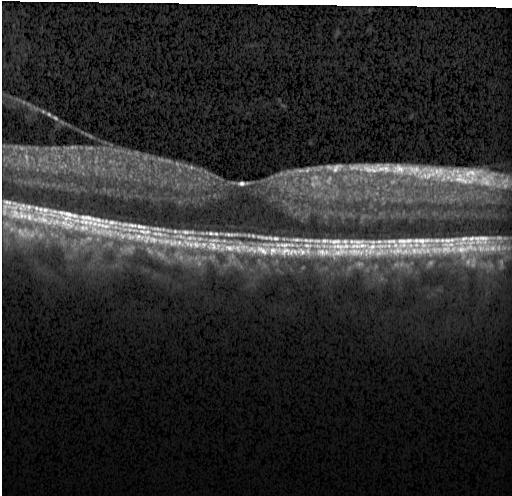

Impression: no choroidal neovascularization, no diabetic macular edema, and no drusen.